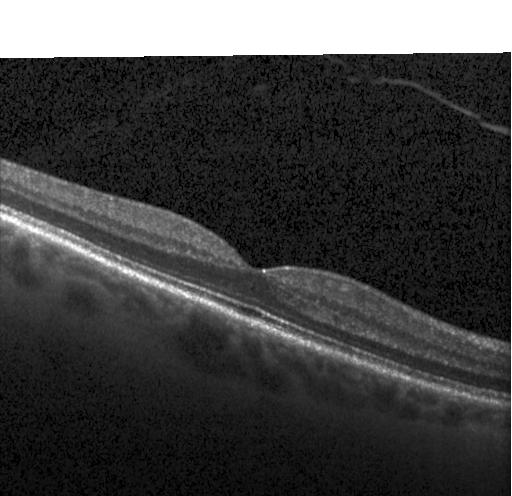 Retinal OCT B-scan. Impression: no choroidal neovascularization, diabetic macular edema, or drusen.